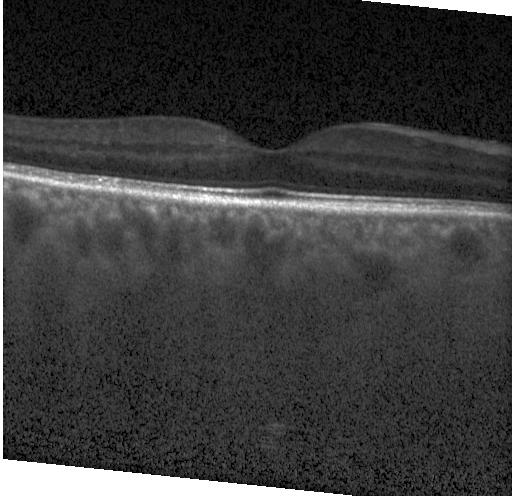

Macular OCT demonstrating no evidence of CNV, DME, or drusen.